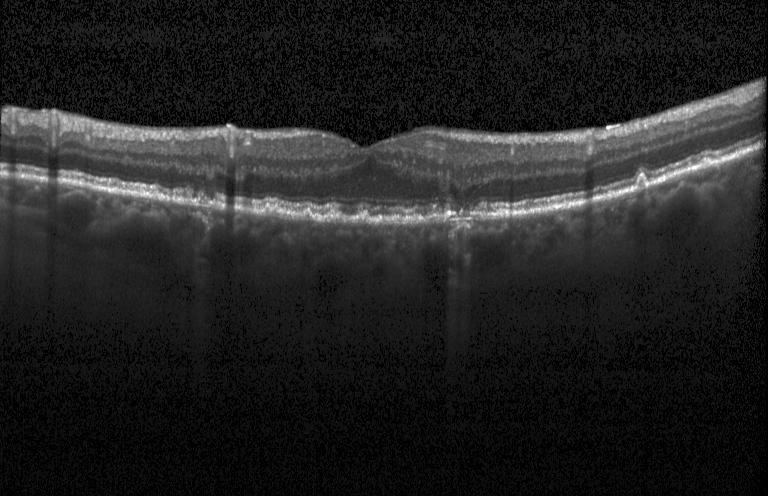

Macular OCT: multiple drusen.